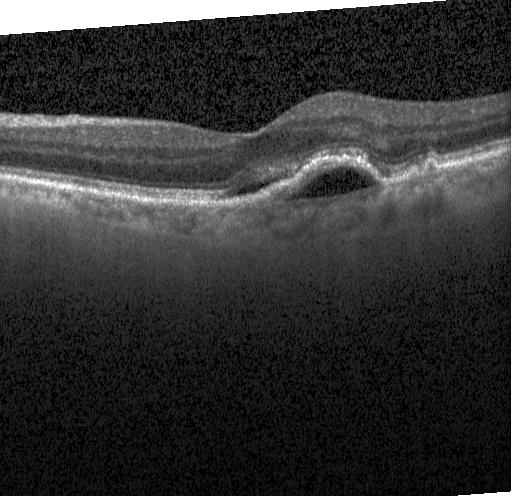
Optical coherence tomography scan · centered on the fovea — OCT finding: choroidal neovascularization (CNV).